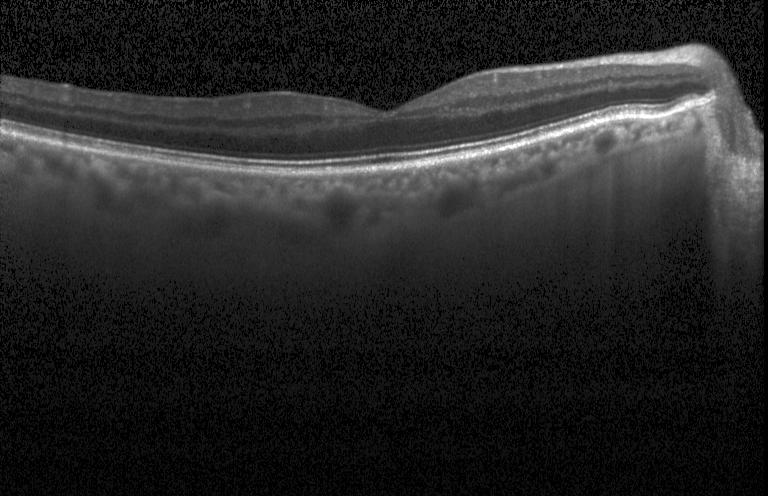
Instrument: Heidelberg Spectralis; OCT B-scan; SD-OCT.
This B-scan demonstrates no choroidal neovascularization, diabetic macular edema, or drusen.